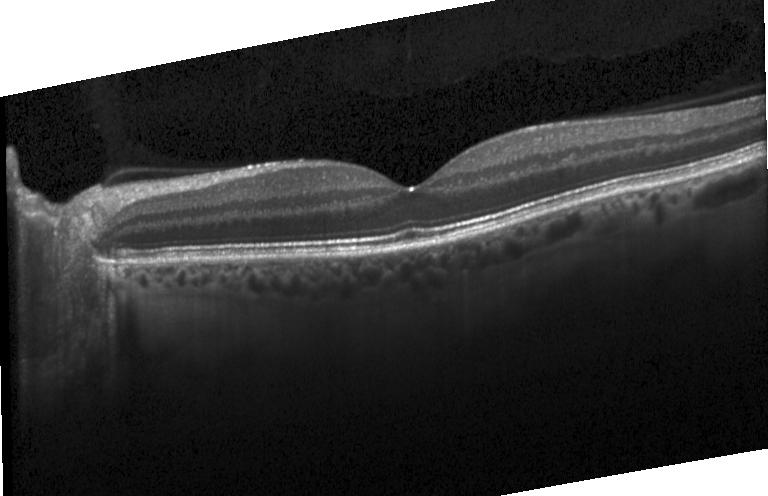
Optical coherence tomography B-scan; SD-OCT
Impression: no evidence of choroidal neovascularization, diabetic macular edema, or drusen.